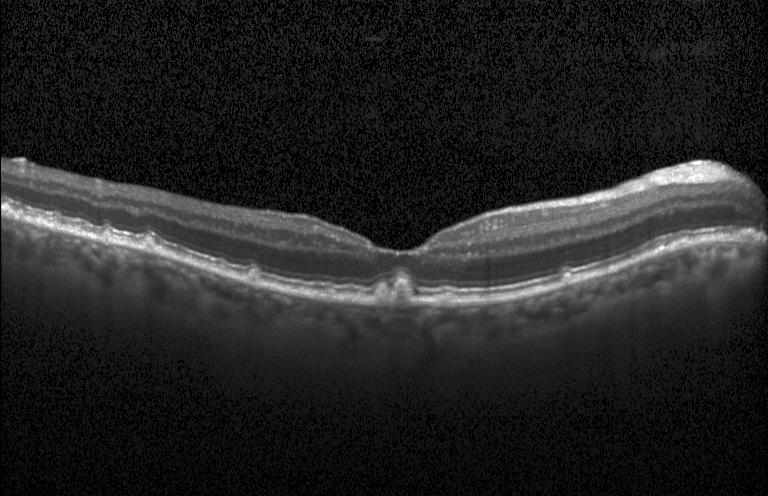

Assessment: drusen.